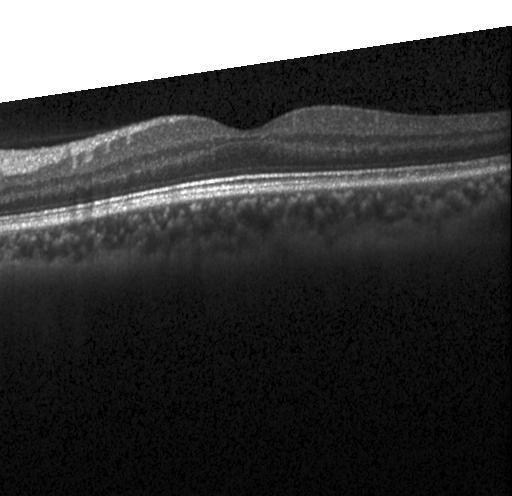 SD-OCT. Fovea-centered. Heidelberg Spectralis. OCT B-scan — No choroidal neovascularization, no diabetic macular edema, and no drusen.